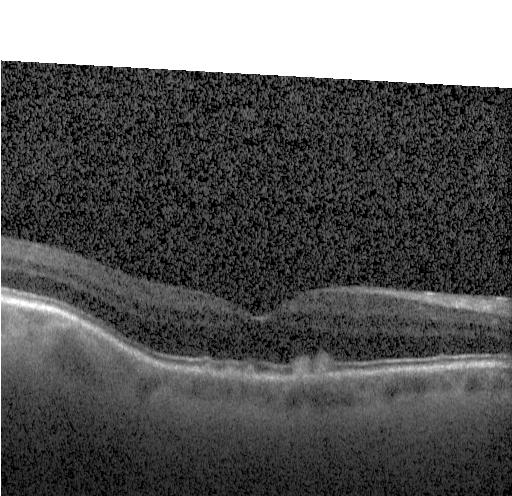
Centered on the fovea; retinal OCT B-scan. The scan shows drusen.